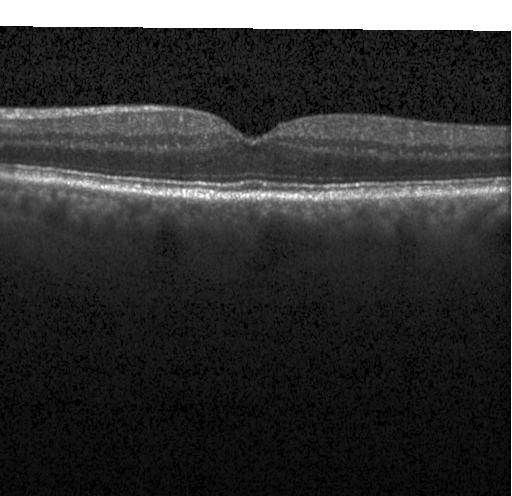

Diagnosis: no evidence of CNV, DME, or drusen.